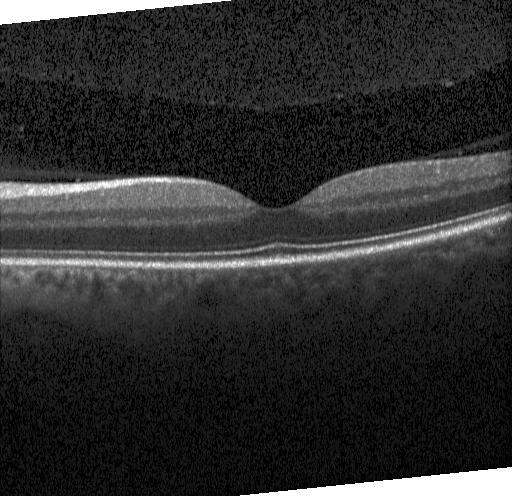 Optical coherence tomography scan · horizontal scan through the fovea.
The scan shows no choroidal neovascularization, no diabetic macular edema, and no drusen.